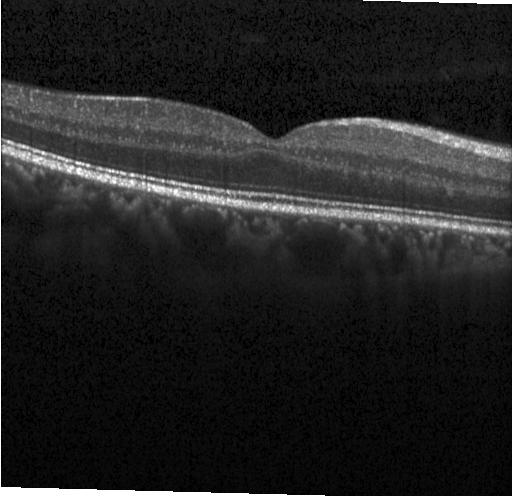 Retinal OCT cross-section showing no CNV, DME, or drusen.